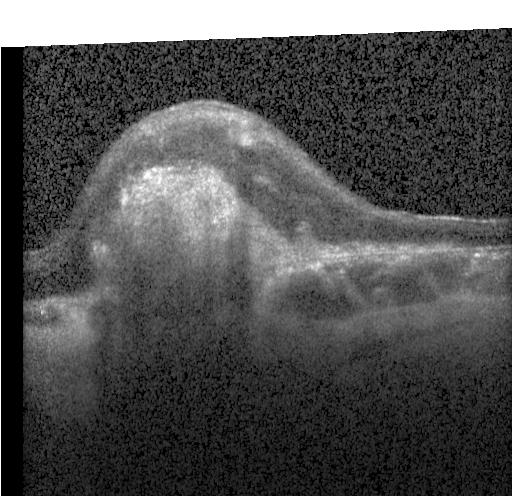 Spectral-domain OCT. Centered on the fovea. Retinal OCT B-scan. Heidelberg Spectralis OCT system
Dx: a choroidal neovascular membrane.